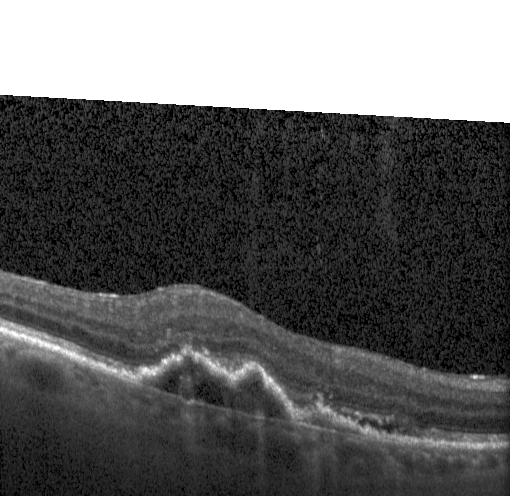 SD-OCT; optical coherence tomography scan. The scan shows a choroidal neovascular membrane.